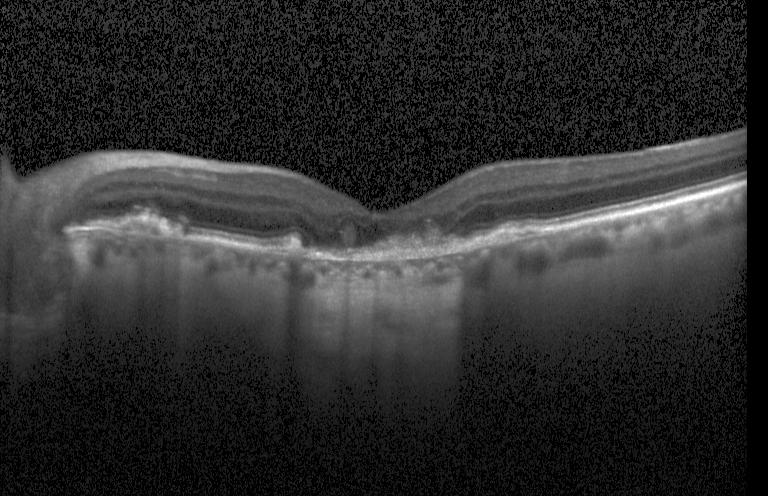

Fovea-centered · optical coherence tomography B-scan
Impression: choroidal neovascularization (CNV).